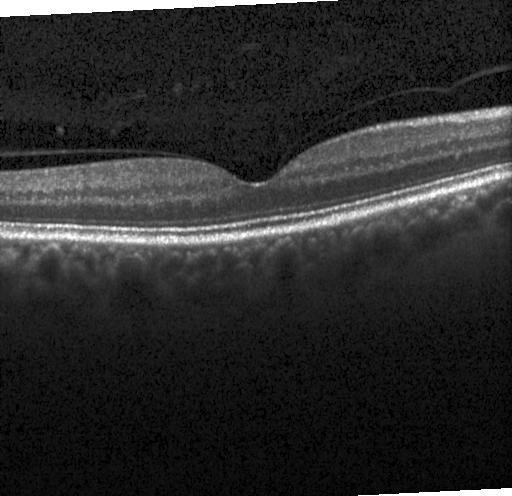 Heidelberg Spectralis, optical coherence tomography scan, horizontal scan through the fovea, spectral-domain OCT. Dx: no choroidal neovascularization, diabetic macular edema, or drusen.